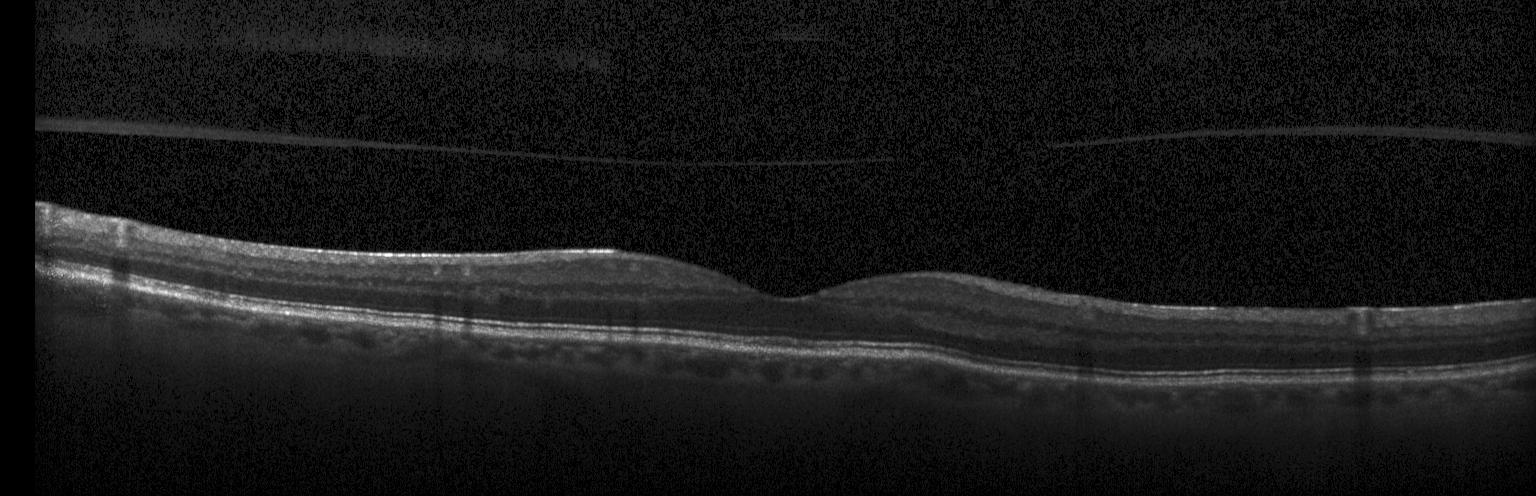
Impression: no evidence of choroidal neovascularization, diabetic macular edema, or drusen.